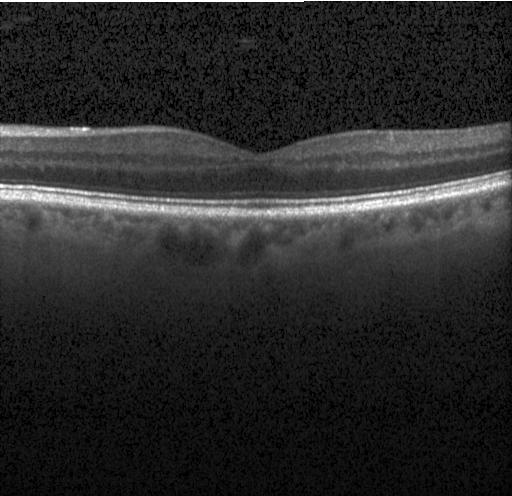
Optical coherence tomography scan — Neither CNV, DME, nor drusen.